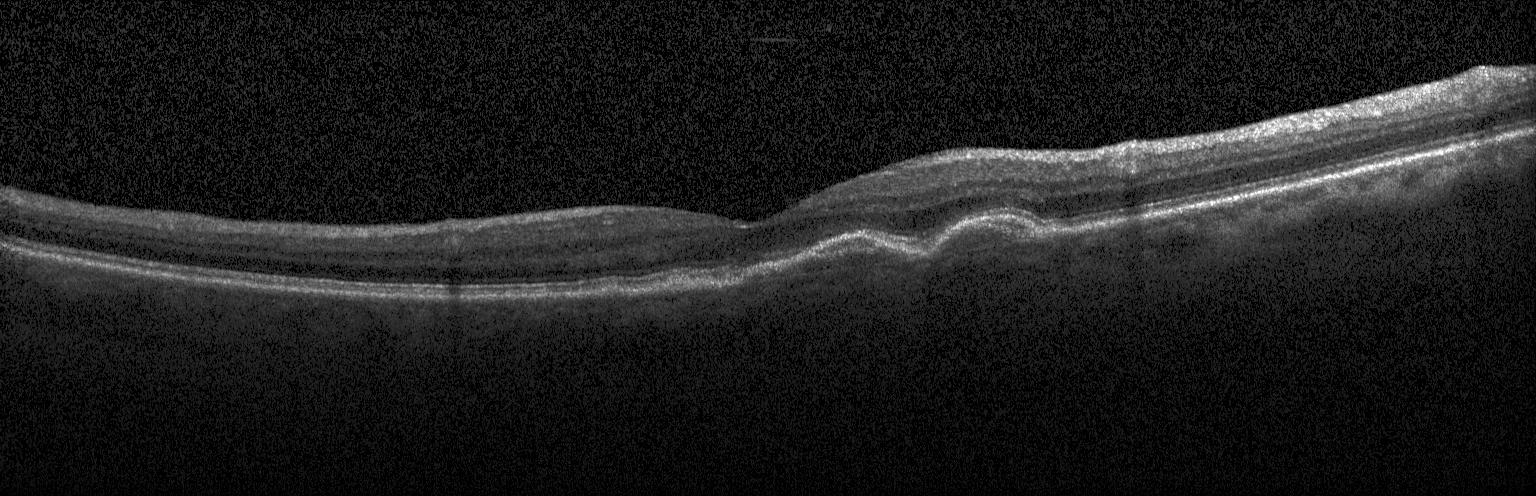
Macular OCT: CNV.